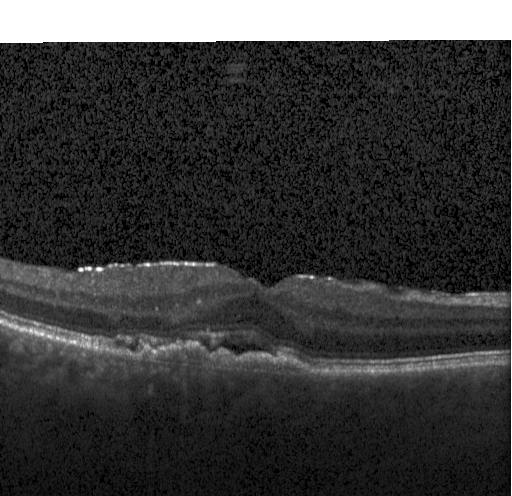

Assessment: choroidal neovascularization.